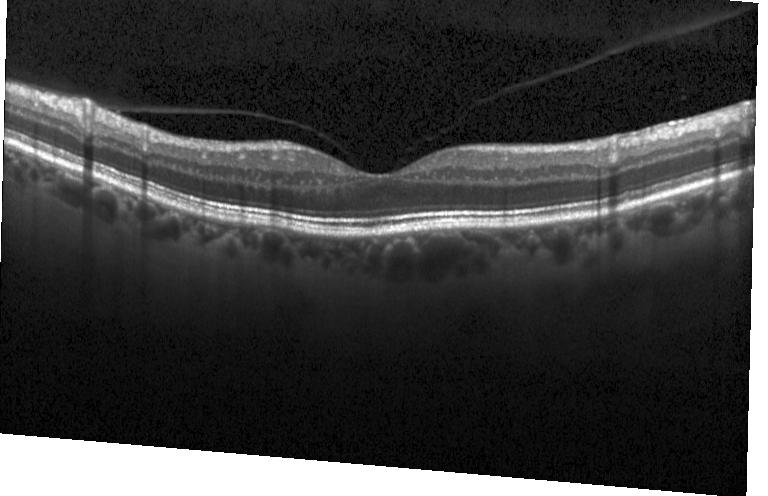 Horizontal scan through the fovea. SD-OCT. Retinal OCT B-scan. Instrument: Heidelberg Spectralis.
Diagnosis: neither CNV, DME, nor drusen.